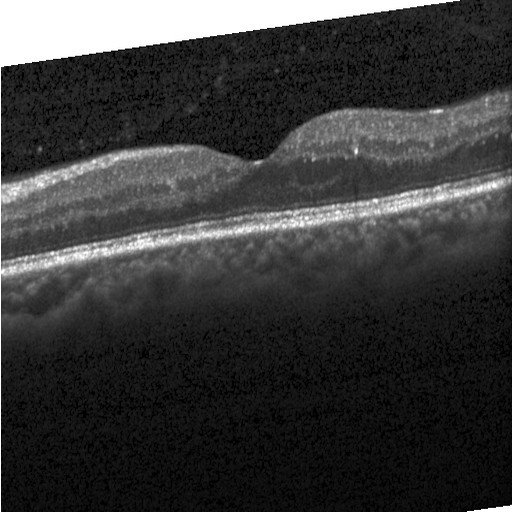 OCT finding: diabetic macular edema (DME).